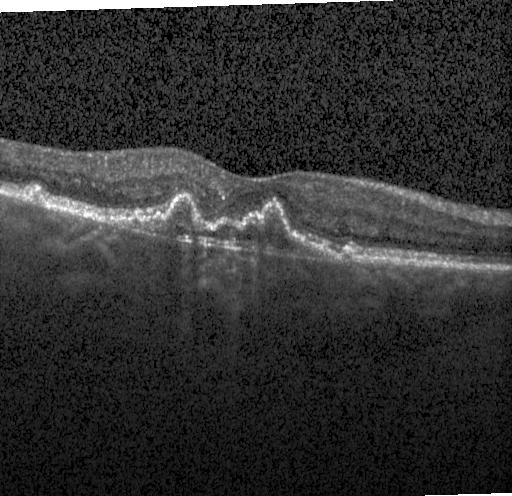
SD-OCT, retinal OCT cross-section, instrument: Heidelberg Spectralis, fovea-centered. OCT finding: a choroidal neovascular membrane.